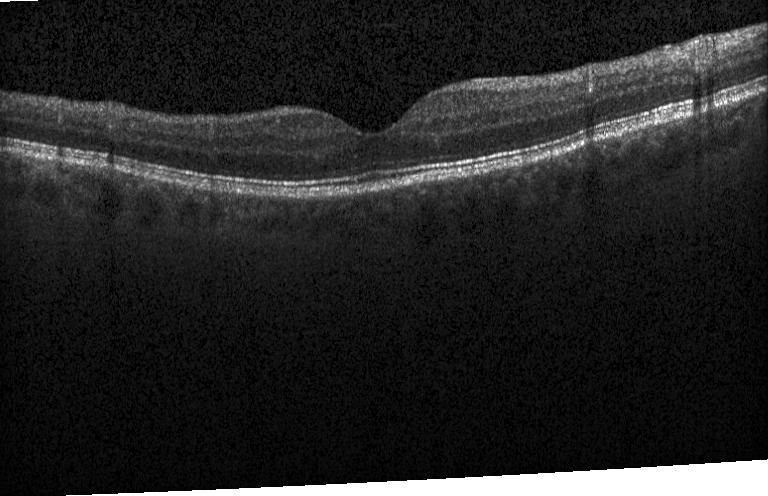 OCT B-scan — This B-scan demonstrates no CNV, DME, or drusen.